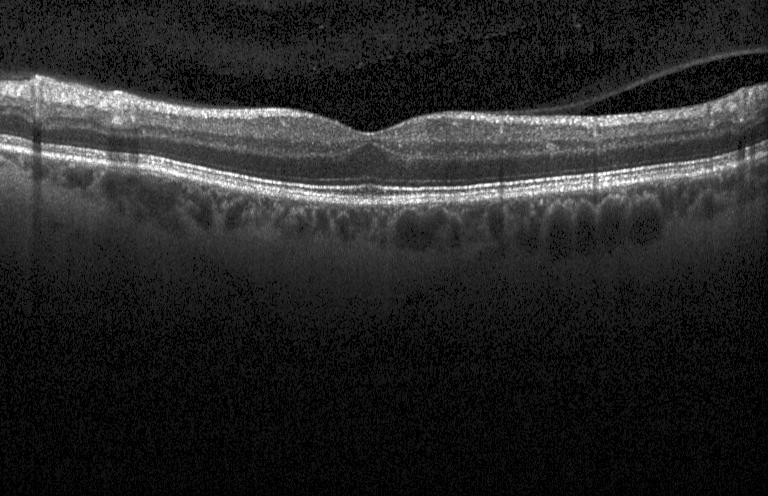
Retinal OCT B-scan — This B-scan demonstrates neither choroidal neovascularization, diabetic macular edema, nor drusen.